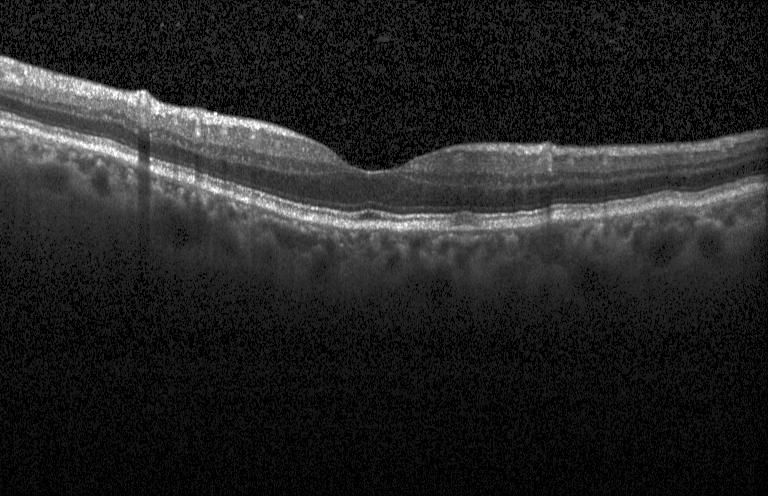
Retinal OCT B-scan. SD-OCT. Instrument: Heidelberg Spectralis
Finding: no choroidal neovascularization, diabetic macular edema, or drusen.